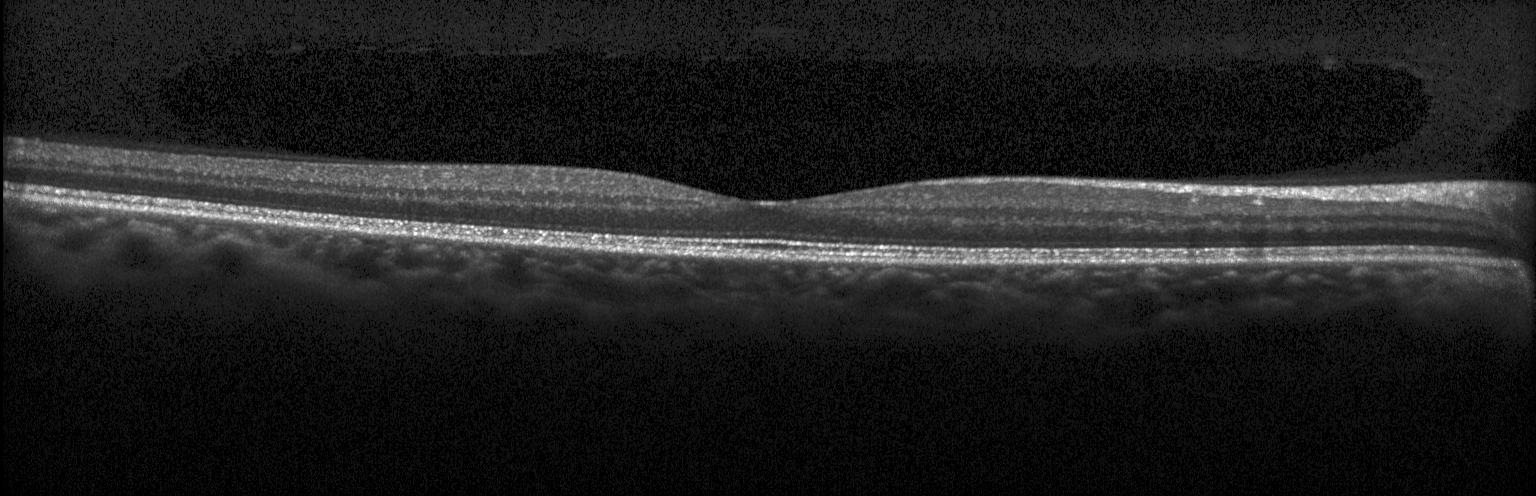 OCT B-scan, acquired on a Heidelberg Spectralis, fovea-centered. This B-scan demonstrates neither CNV, DME, nor drusen.